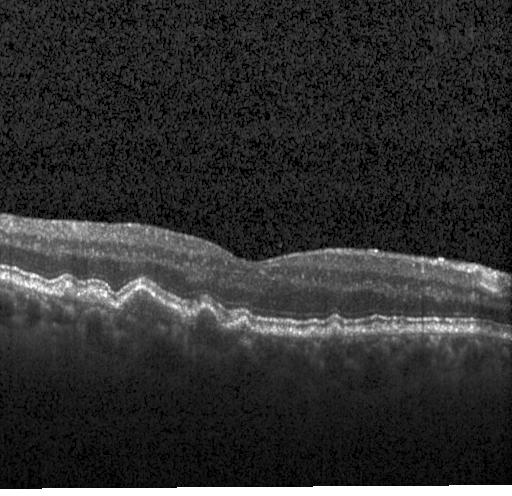
Fovea-centered. OCT line scan. SD-OCT.
Diagnosis: multiple drusen.